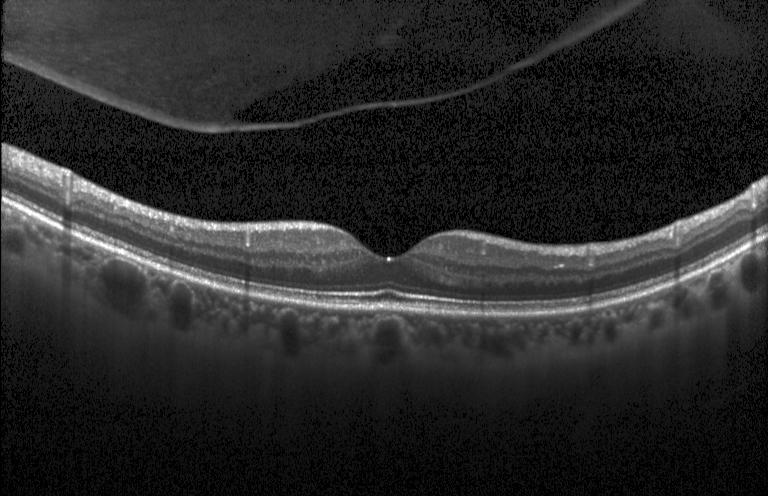 Dx: no evidence of CNV, DME, or drusen.